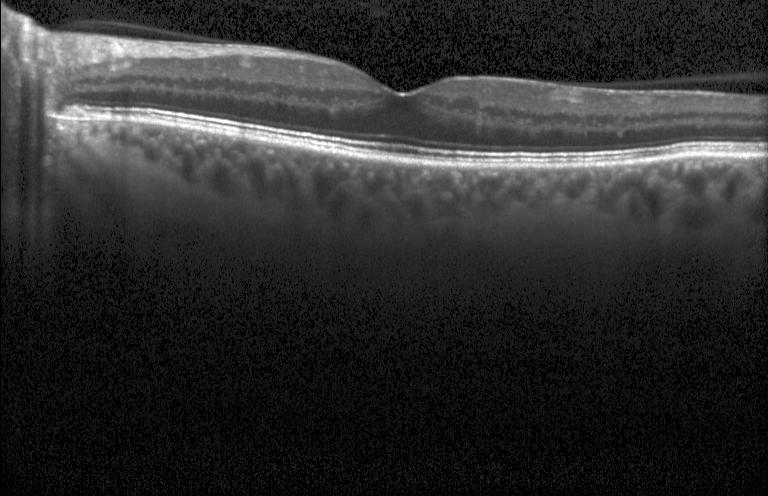

Heidelberg Spectralis; OCT line scan
Macular OCT: no evidence of choroidal neovascularization, diabetic macular edema, or drusen.